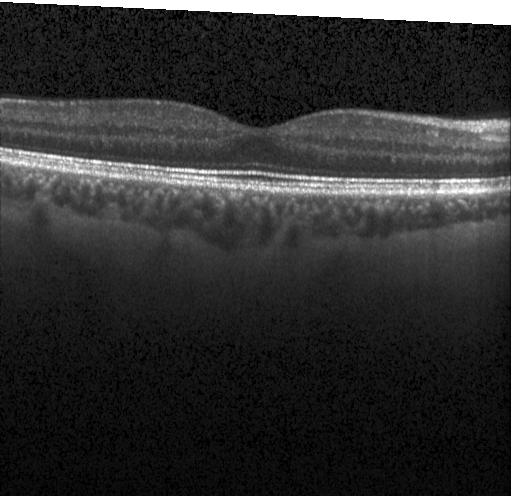 Diagnosis: no choroidal neovascularization, no diabetic macular edema, and no drusen.